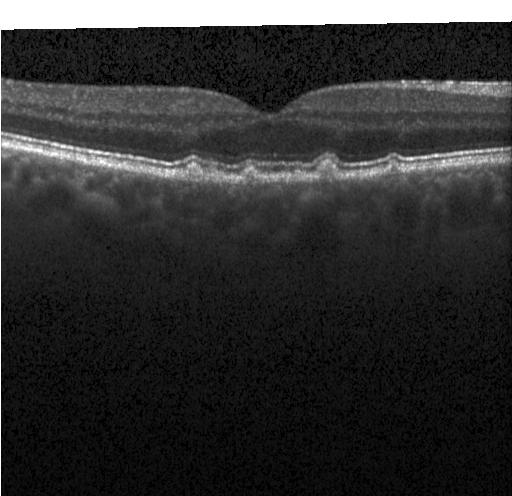

Assessment: sub-RPE drusenoid deposits.